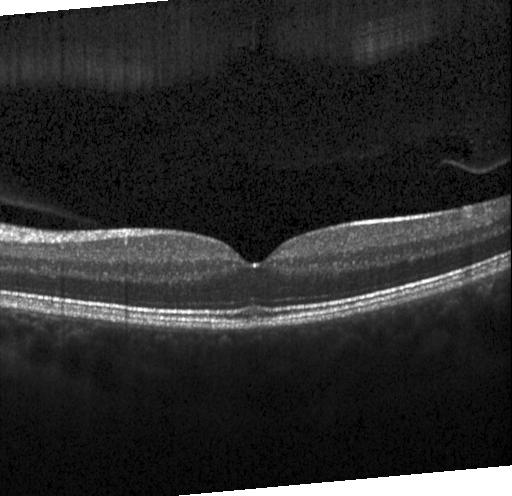

Spectral-domain OCT, retinal OCT cross-section. Diagnosis: neither CNV, DME, nor drusen.